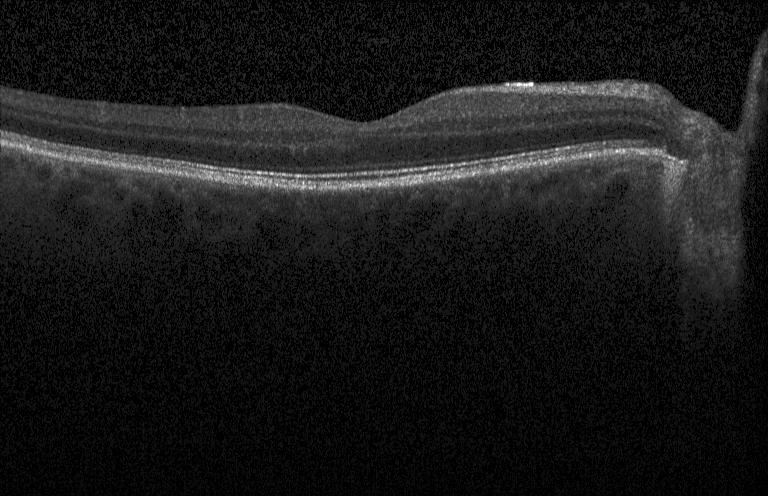

No evidence of CNV, DME, or drusen.